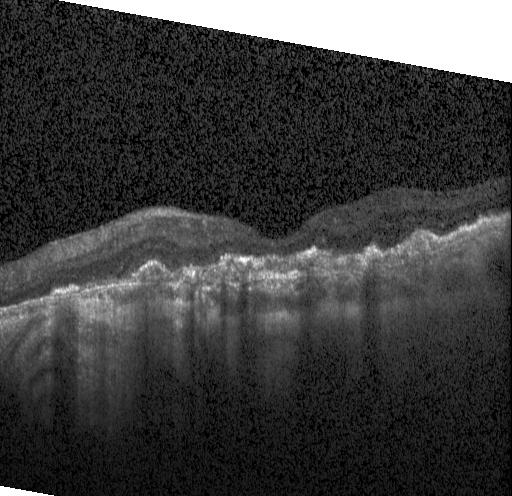 Optical coherence tomography B-scan, spectral-domain optical coherence tomography, through the macula — Finding: choroidal neovascularization.